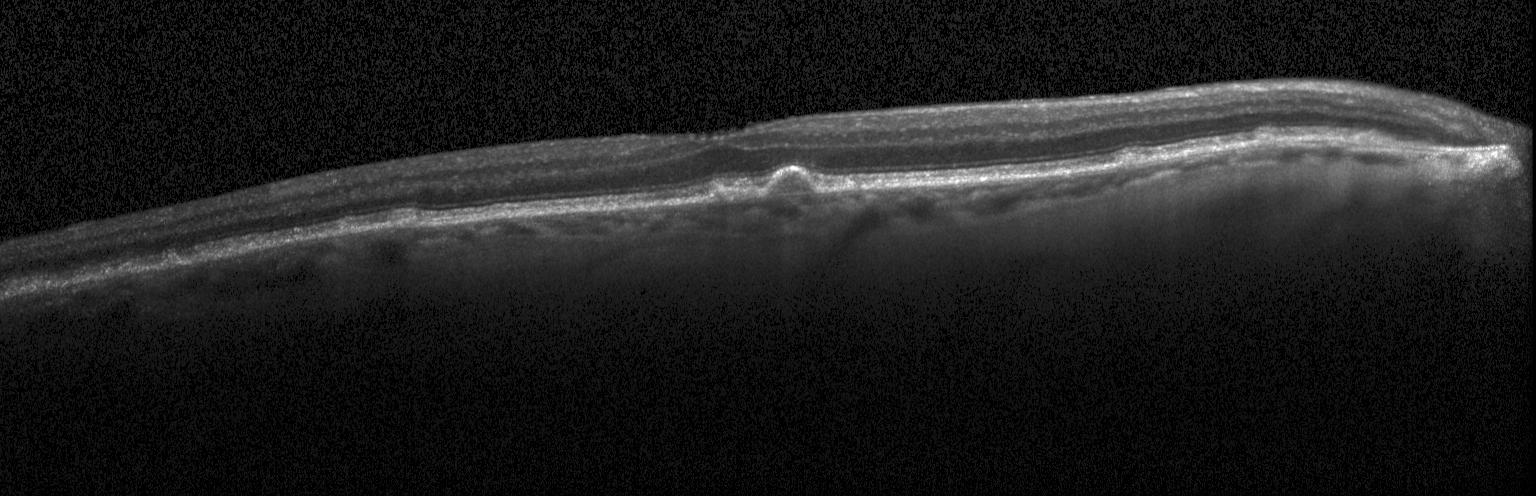 OCT B-scan, fovea-centered.
Dx: multiple drusen.